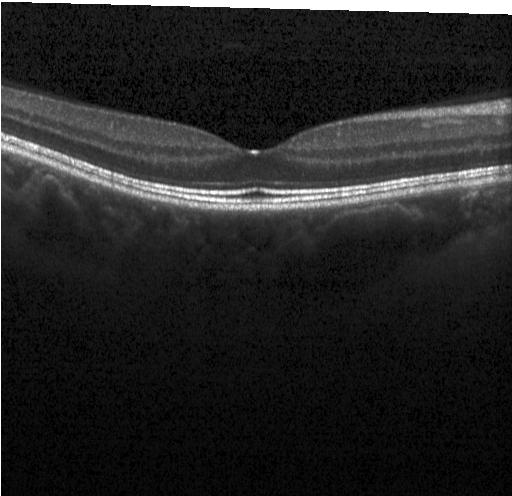

Spectral-domain OCT · retinal OCT B-scan · macular scan.
Finding: no CNV, DME, or drusen.